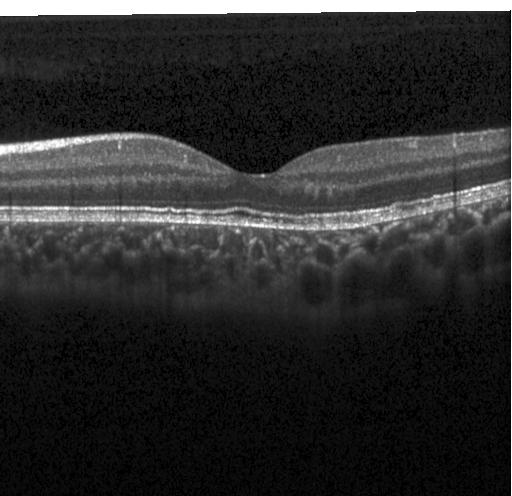

Fovea-centered; optical coherence tomography scan — Diagnosis: no evidence of CNV, DME, or drusen.